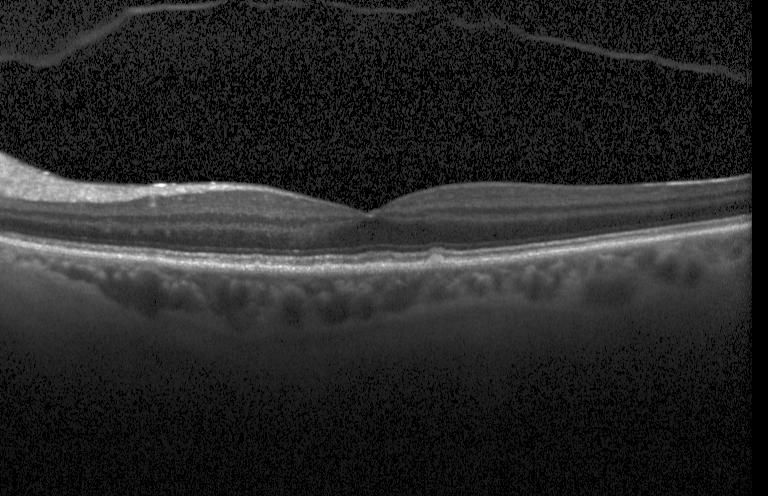 Sub-RPE drusenoid deposits.